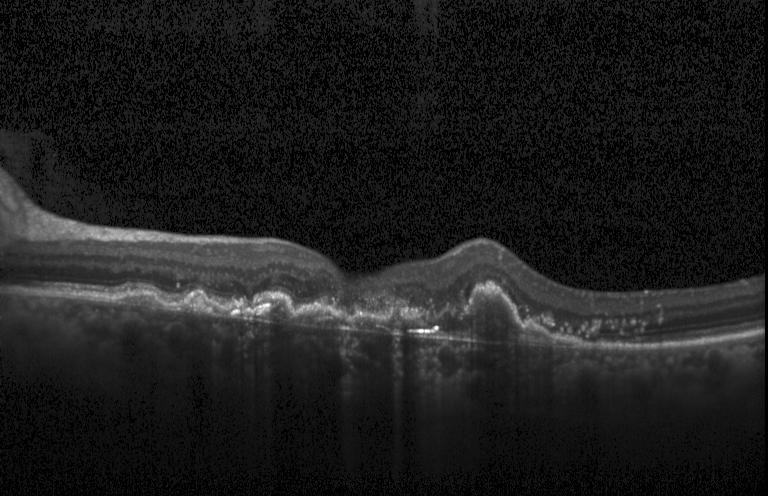 Retinal OCT cross-section showing choroidal neovascularization.